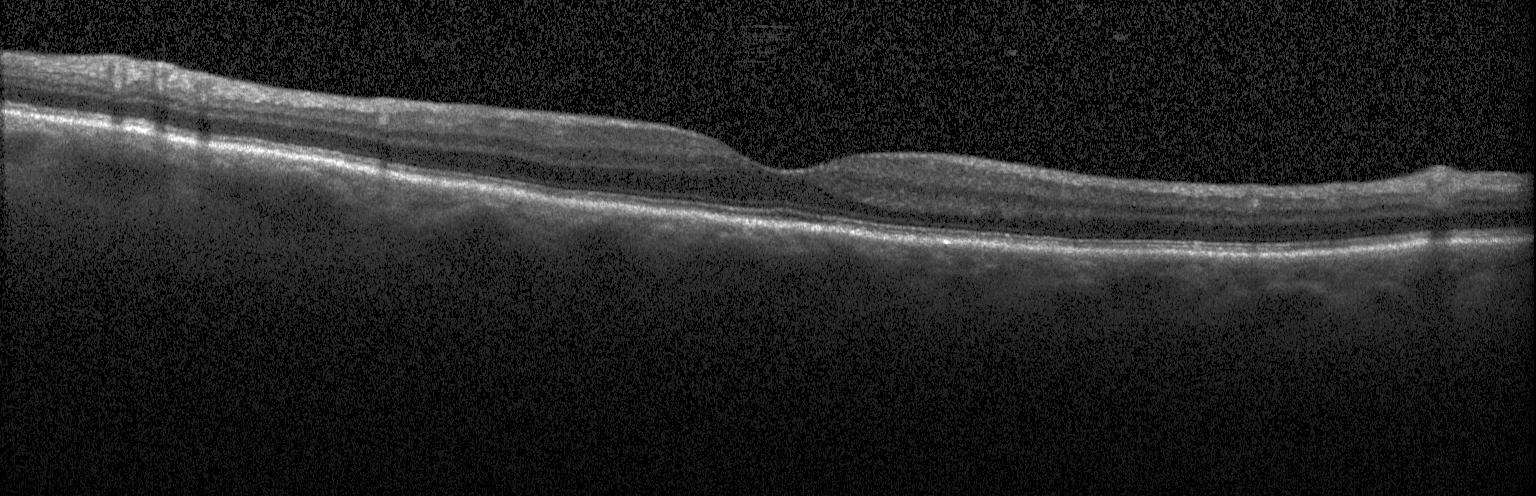 OCT scan showing neither choroidal neovascularization, diabetic macular edema, nor drusen.